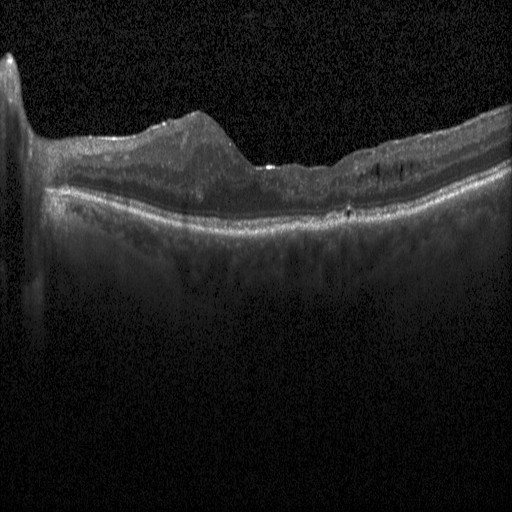 OCT line scan; spectral-domain optical coherence tomography — Diagnosis: diabetic macular edema.